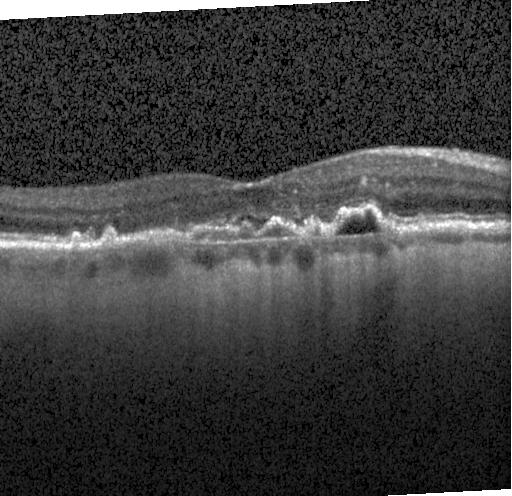

SD-OCT, acquired on a Heidelberg Spectralis, OCT B-scan, through the macula — Impression: a choroidal neovascular membrane.